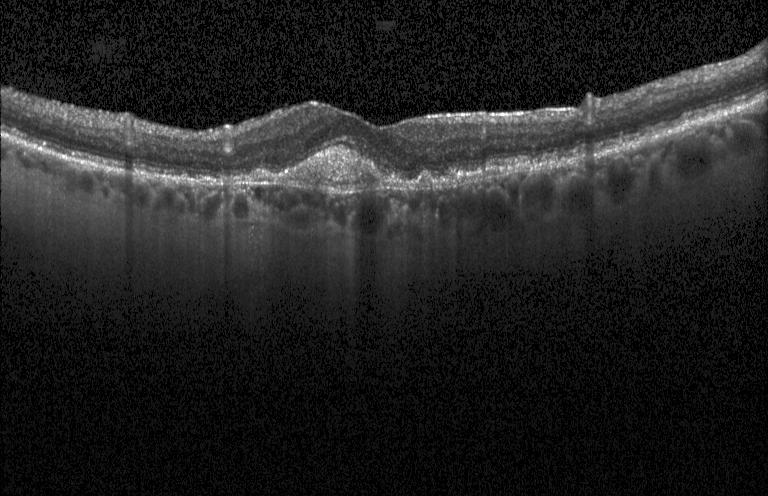
Spectral-domain OCT · optical coherence tomography scan · through the macula — Assessment: a choroidal neovascular membrane.